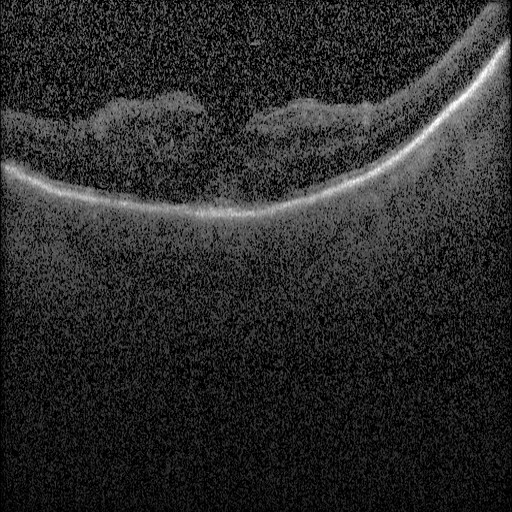

Instrument: Heidelberg Spectralis; OCT B-scan; spectral-domain OCT
Diagnosis: diabetic macular edema (DME).